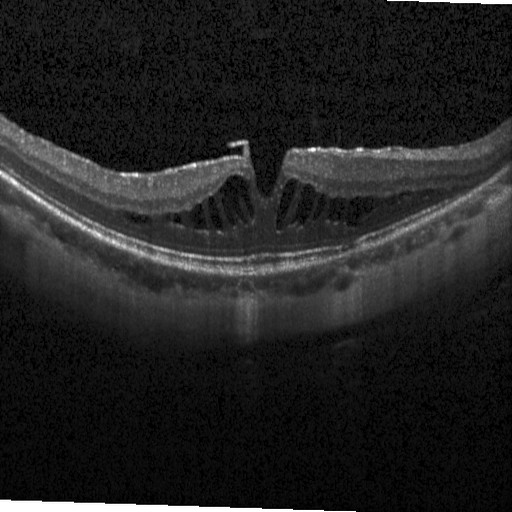

Instrument: Heidelberg Spectralis; retinal OCT cross-section; through the macula.
Finding: diabetic macular edema.